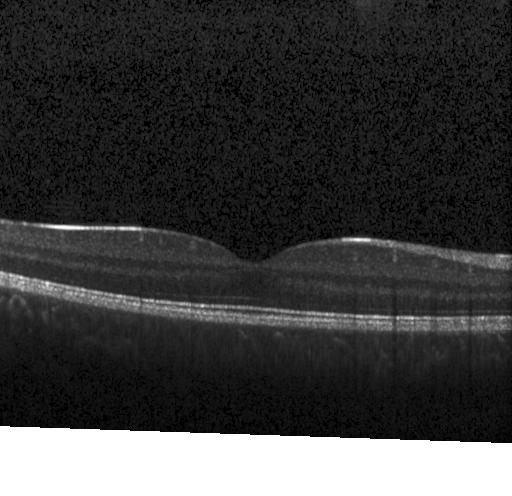

Heidelberg Spectralis. Retinal OCT cross-section
The scan shows neither CNV, DME, nor drusen.